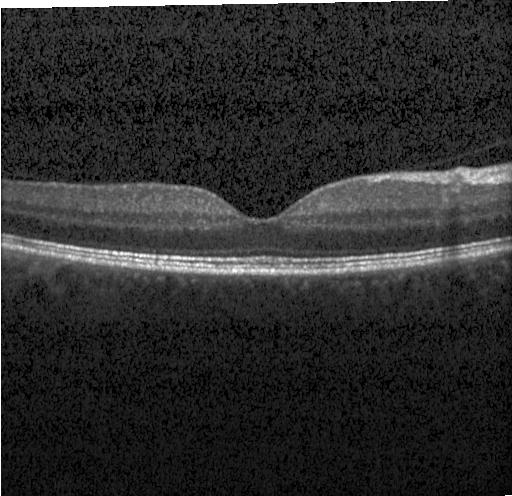

OCT finding: neither CNV, DME, nor drusen.